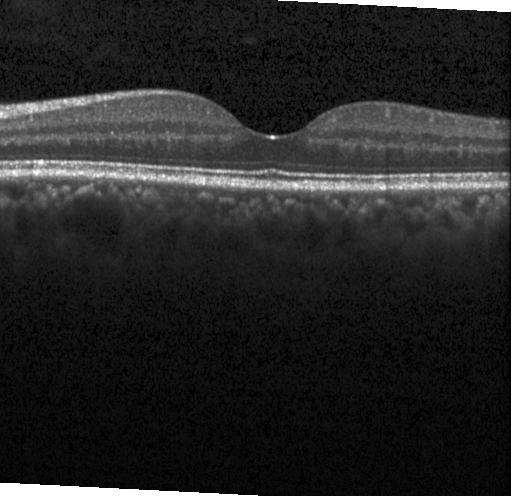
OCT B-scan. Fovea-centered. SD-OCT — Impression: no CNV, DME, or drusen.